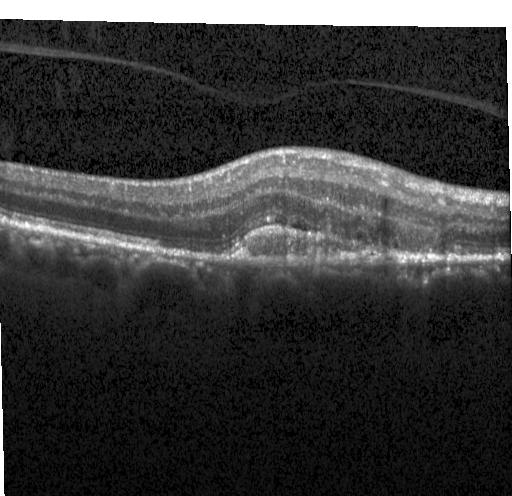
Spectral-domain OCT B-scan: a choroidal neovascular membrane.